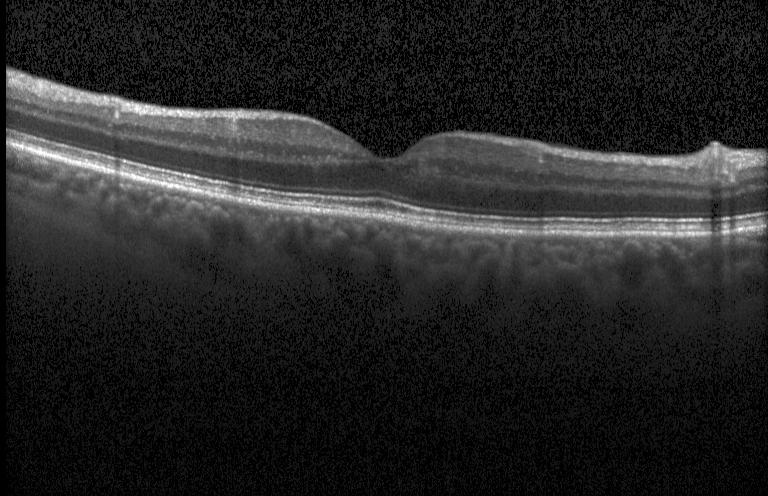

Spectral-domain optical coherence tomography · OCT line scan · Heidelberg Spectralis OCT system · through the macula
This B-scan demonstrates no evidence of choroidal neovascularization, diabetic macular edema, or drusen.